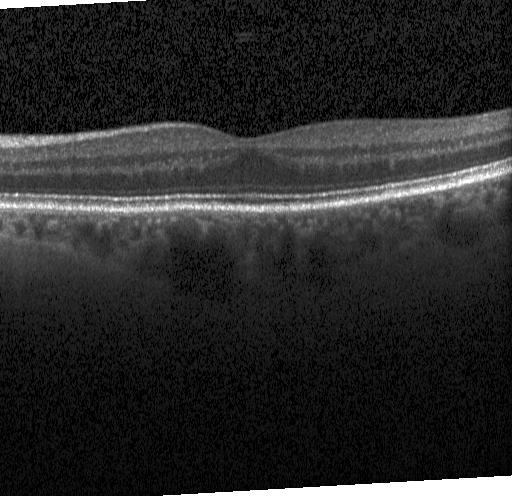
Horizontal scan through the fovea · OCT B-scan · instrument: Heidelberg Spectralis · spectral-domain OCT
Diagnosis: neither CNV, DME, nor drusen.